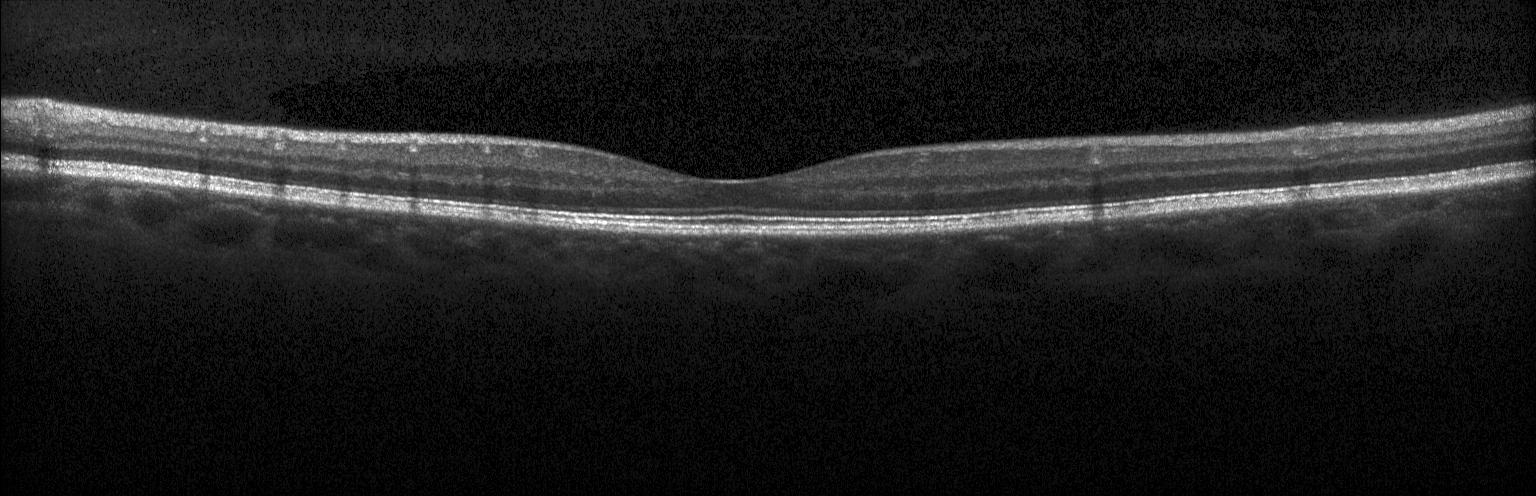
Impression: no choroidal neovascularization, no diabetic macular edema, and no drusen.